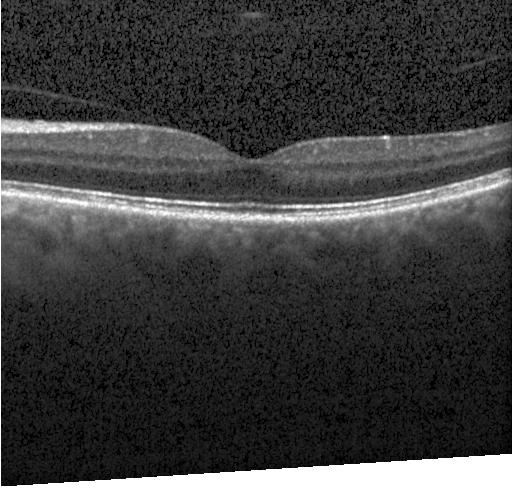 Instrument: Heidelberg Spectralis; retinal OCT cross-section; horizontal scan through the fovea; SD-OCT — The scan shows no choroidal neovascularization, no diabetic macular edema, and no drusen.